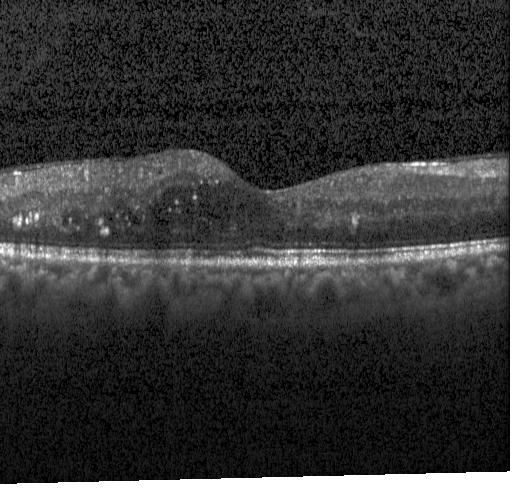 Dx: DME.